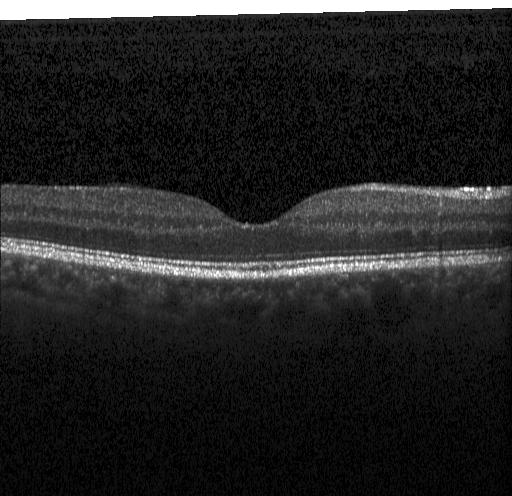
Horizontal scan through the fovea, Heidelberg Spectralis, OCT B-scan. Impression: no evidence of choroidal neovascularization, diabetic macular edema, or drusen.